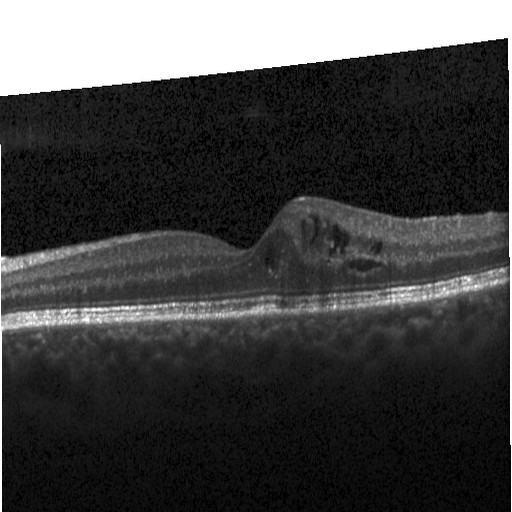 OCT B-scan, SD-OCT, Heidelberg Spectralis OCT system, horizontal scan through the fovea. Finding: diabetic macular edema.